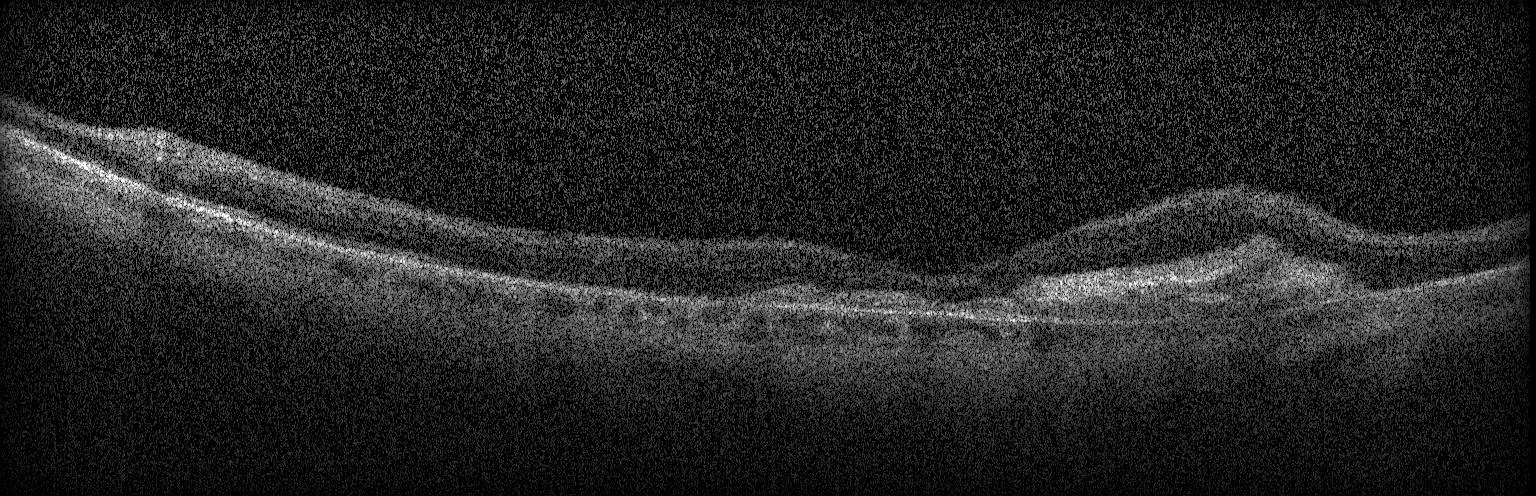 Spectral-domain optical coherence tomography. Acquired on a Heidelberg Spectralis. Retinal OCT B-scan. Finding: a choroidal neovascular membrane.